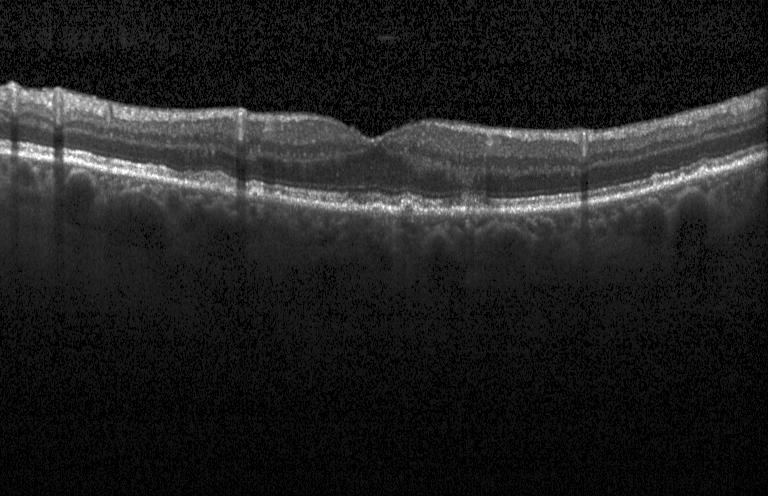

Diagnosis: drusen.